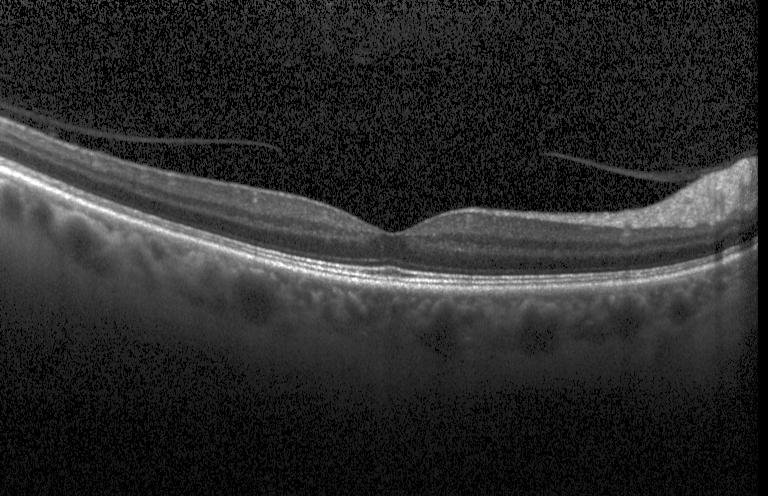 Retinal OCT B-scan.
This B-scan demonstrates no CNV, DME, or drusen.